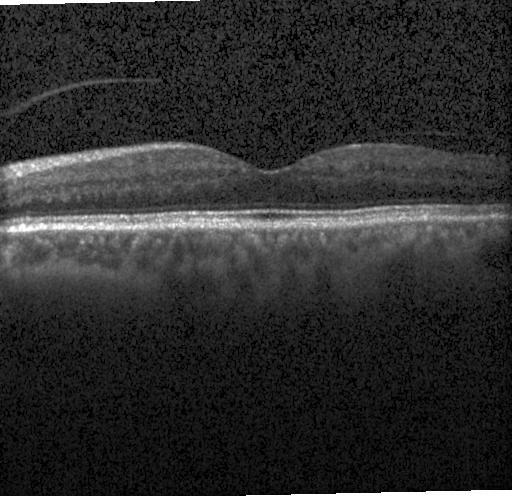
Diagnosis: no choroidal neovascularization, no diabetic macular edema, and no drusen.